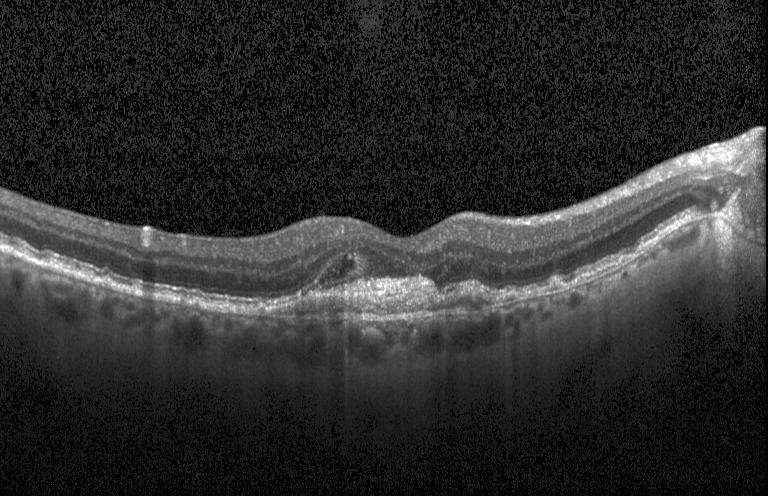
Retinal OCT B-scan. Impression: CNV.